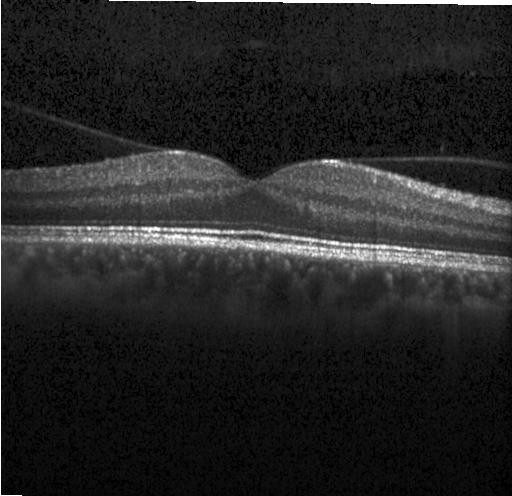
No choroidal neovascularization, no diabetic macular edema, and no drusen.